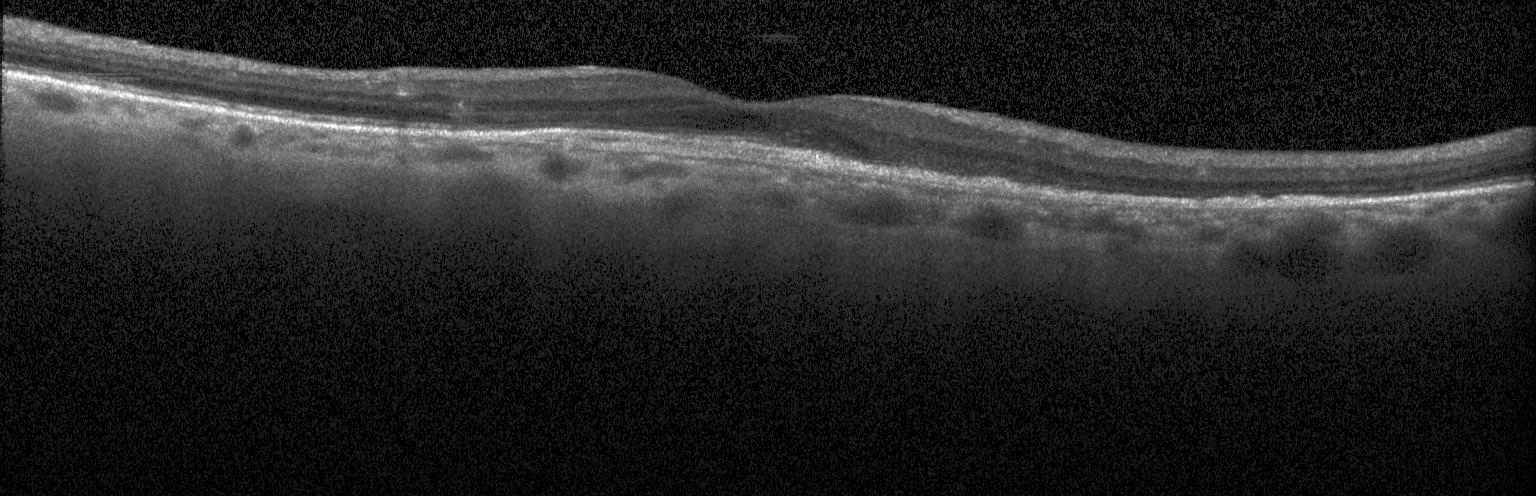

Spectral-domain OCT; OCT line scan; macular scan.
Finding: choroidal neovascularization (CNV).